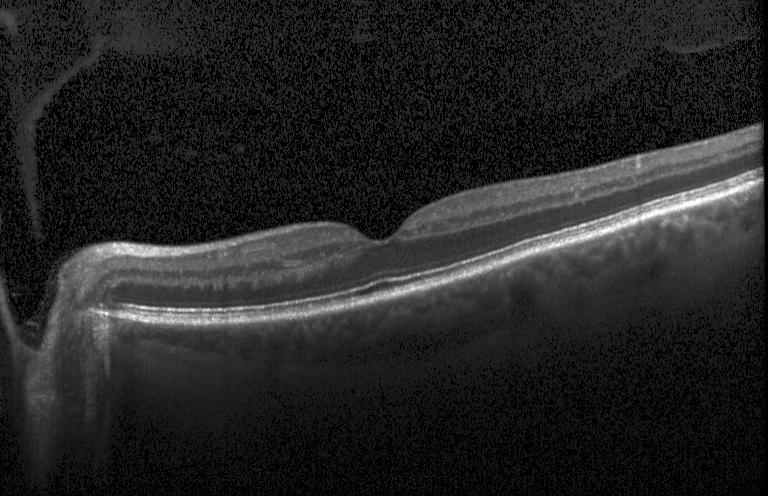
Instrument: Heidelberg Spectralis · optical coherence tomography scan.
Macular OCT: no choroidal neovascularization, no diabetic macular edema, and no drusen.